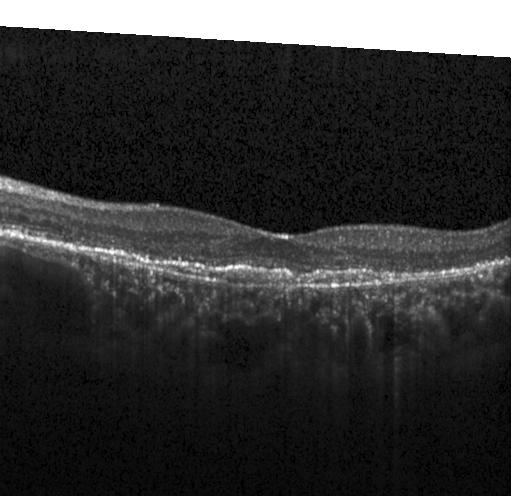 This B-scan demonstrates a choroidal neovascular membrane.